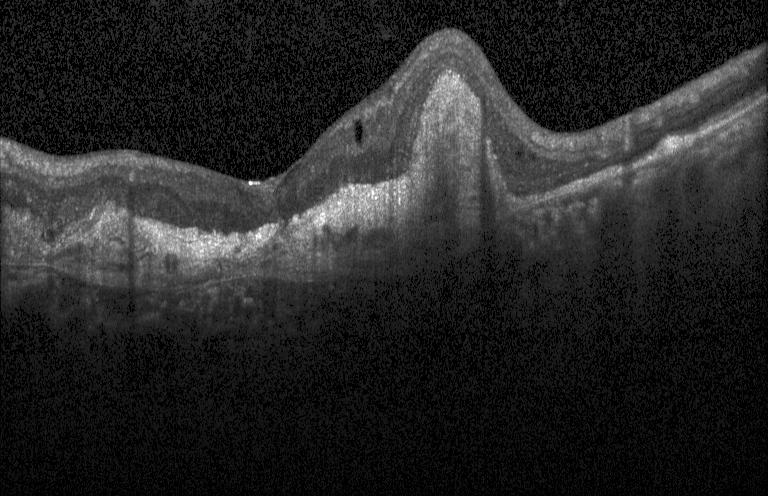 Heidelberg Spectralis OCT system · fovea-centered · OCT line scan. Finding: choroidal neovascularization (CNV).